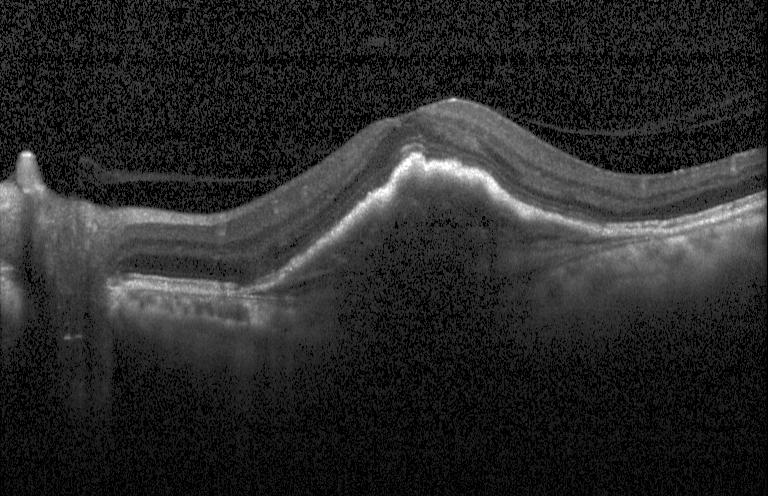
Diagnosis: choroidal neovascularization.